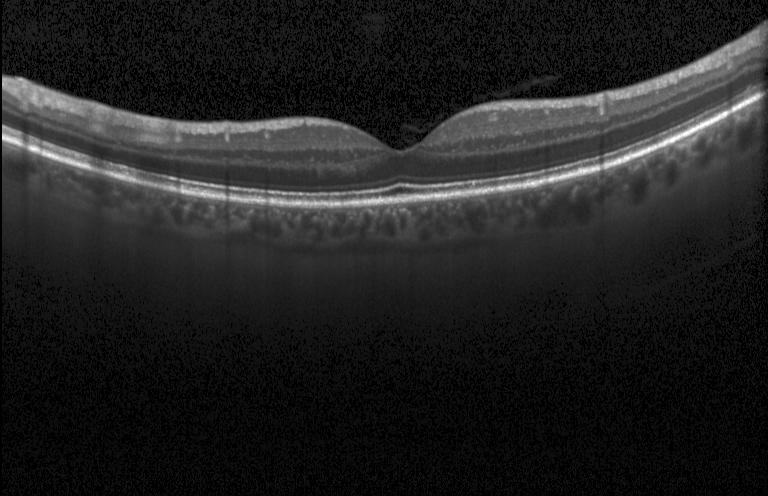

OCT scan showing no choroidal neovascularization, no diabetic macular edema, and no drusen.